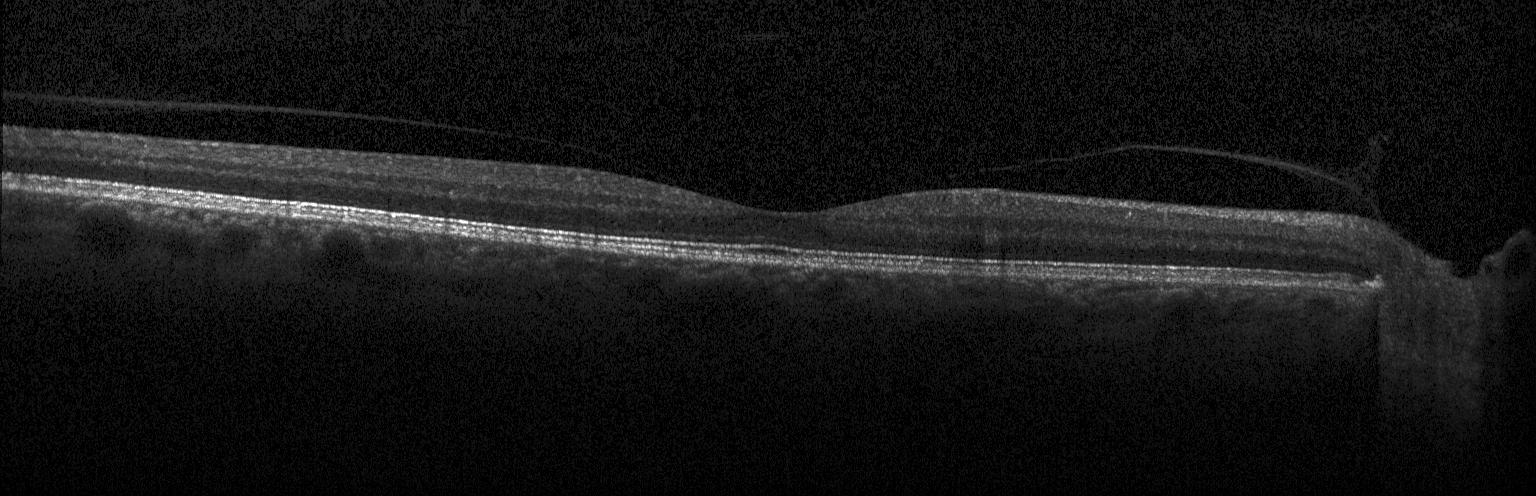
SD-OCT. Optical coherence tomography B-scan.
Dx: no evidence of choroidal neovascularization, diabetic macular edema, or drusen.